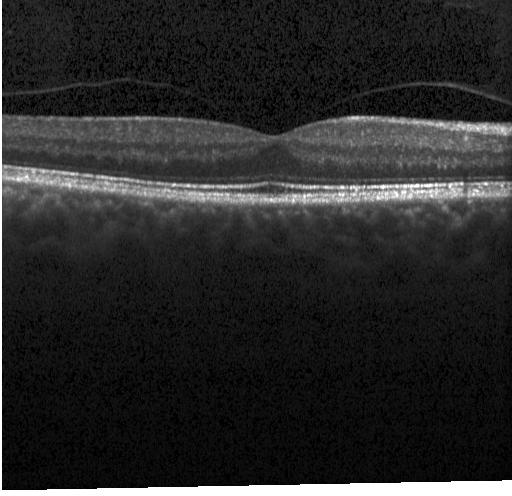
Diagnosis: no evidence of choroidal neovascularization, diabetic macular edema, or drusen.